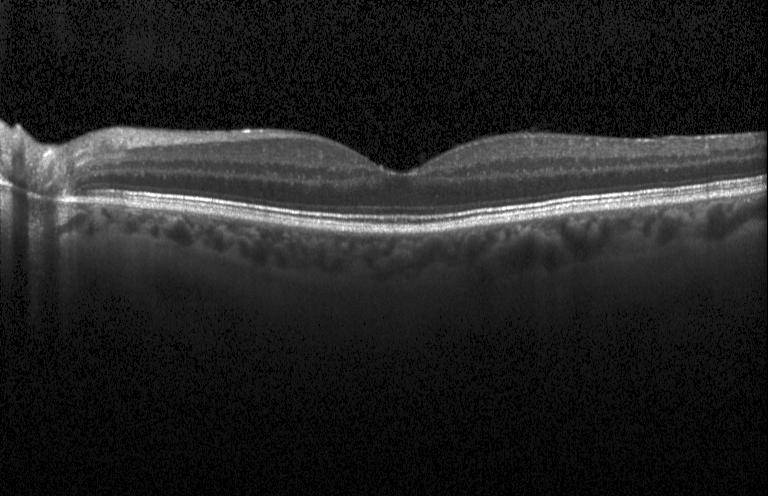

Retinal OCT B-scan.
Finding: no evidence of choroidal neovascularization, diabetic macular edema, or drusen.